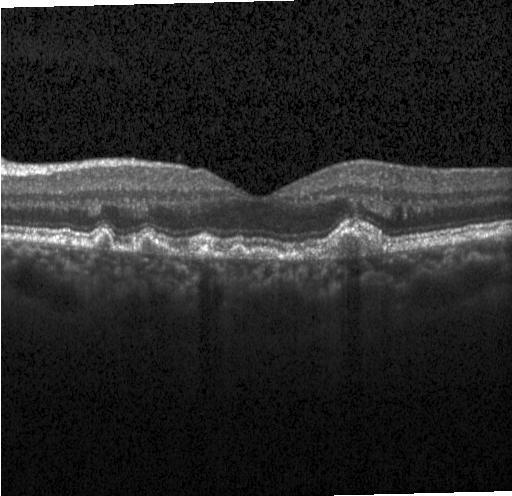
Finding: drusen.